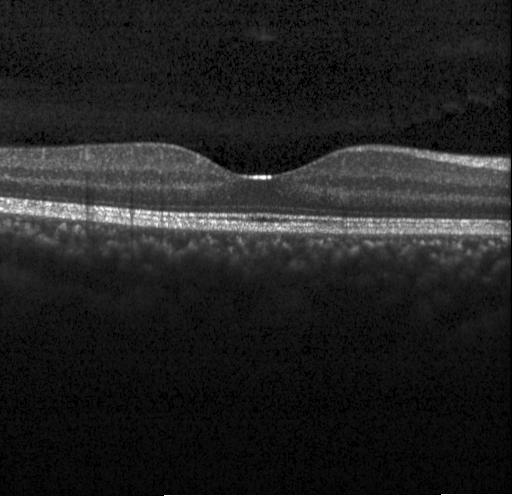 Macular OCT demonstrating neither CNV, DME, nor drusen.